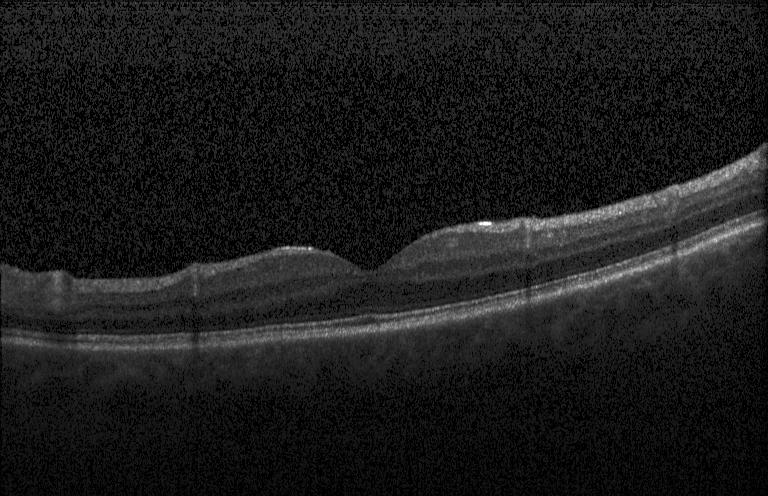 Assessment: neither choroidal neovascularization, diabetic macular edema, nor drusen.